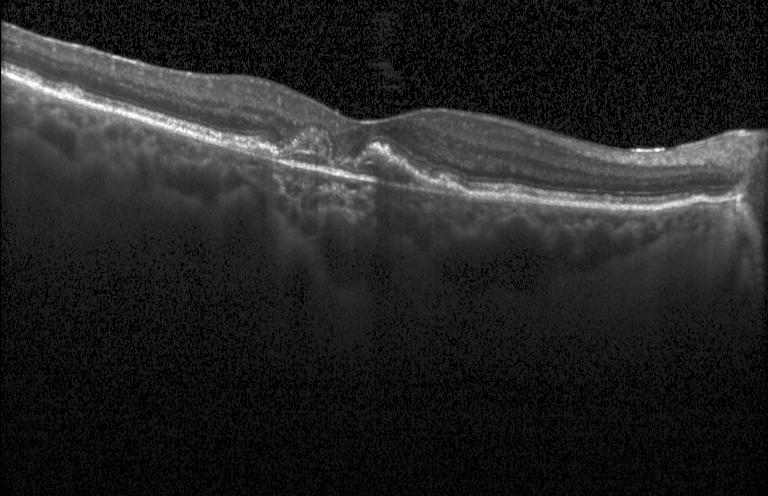
Assessment: choroidal neovascularization.